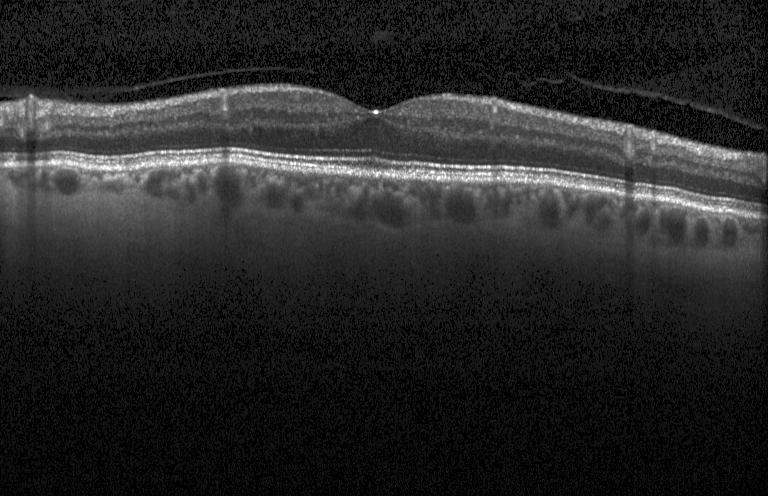 Neither choroidal neovascularization, diabetic macular edema, nor drusen.